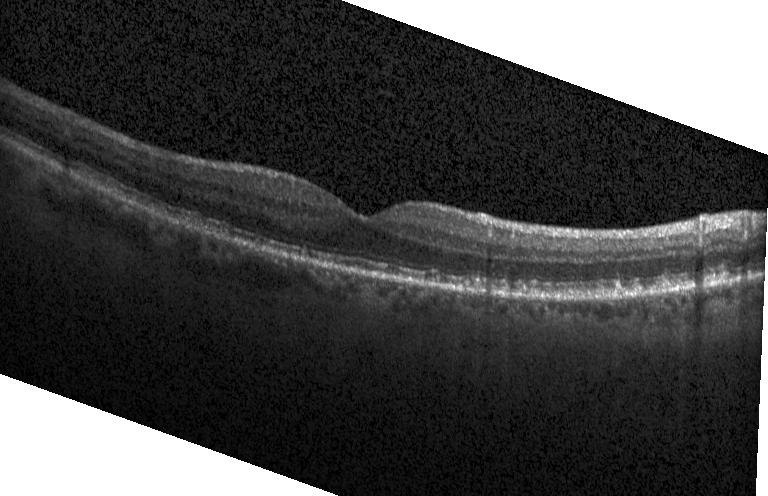 OCT B-scan
Diagnosis: drusen.